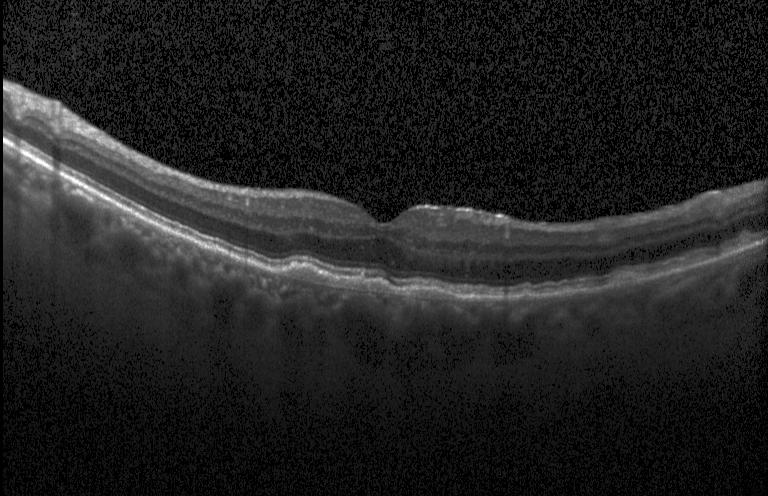
Diagnosis: a choroidal neovascular membrane.